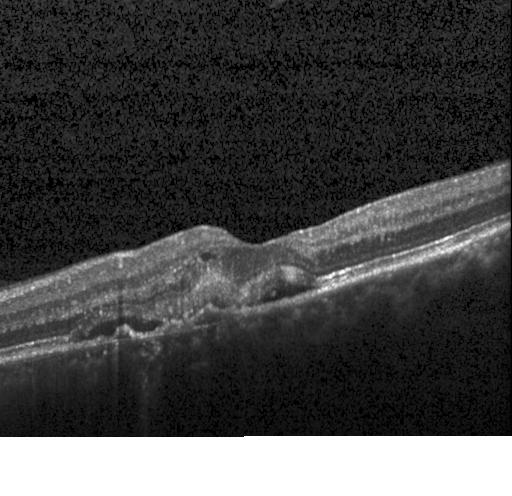

The scan shows choroidal neovascularization.